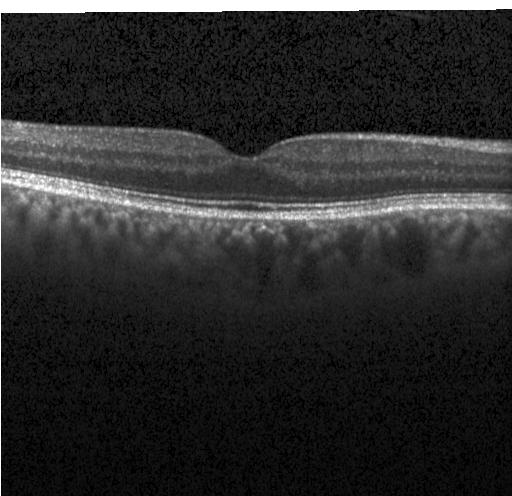
Optical coherence tomography scan
Finding: neither choroidal neovascularization, diabetic macular edema, nor drusen.